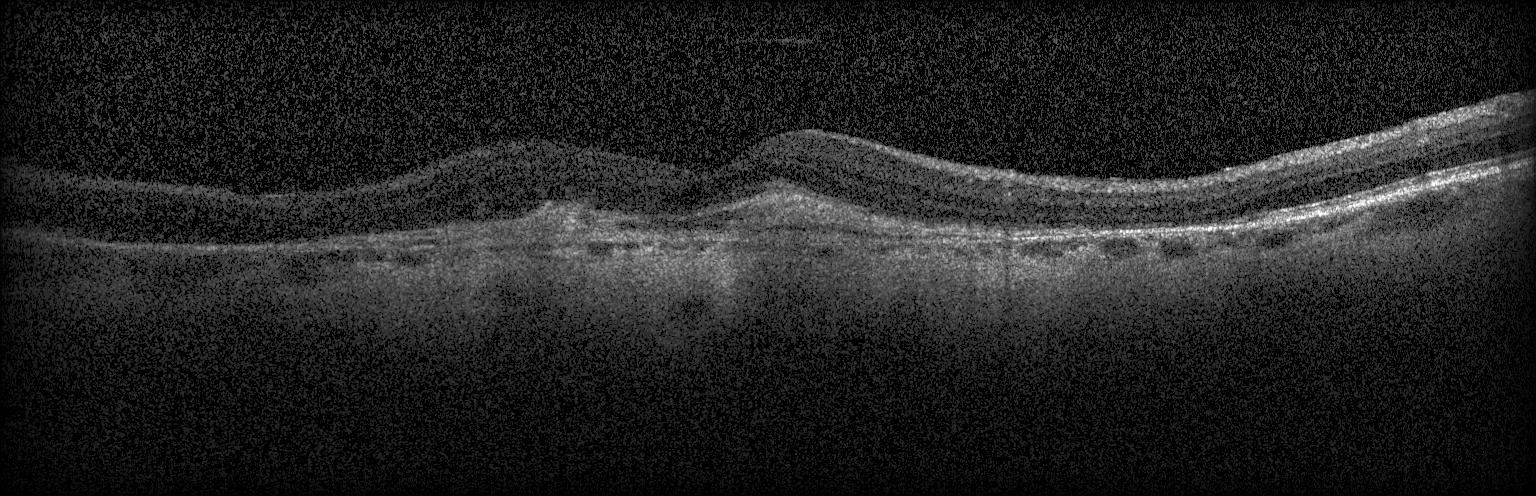

OCT B-scan. Through the macula. Dx: CNV.